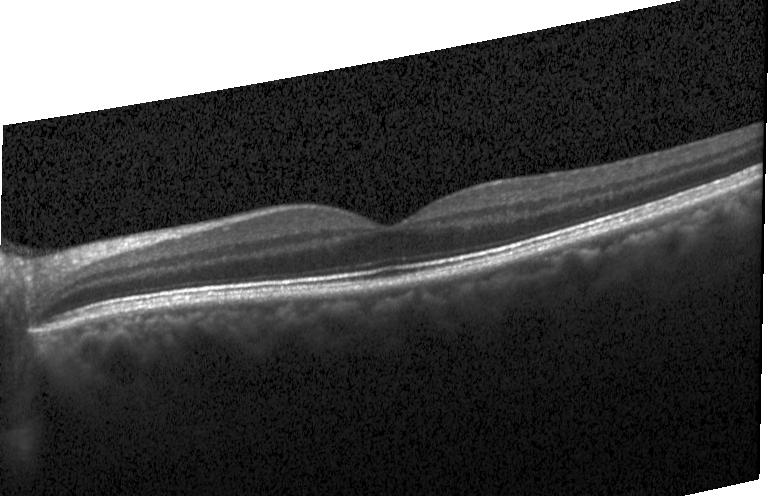 OCT finding: no evidence of choroidal neovascularization, diabetic macular edema, or drusen.